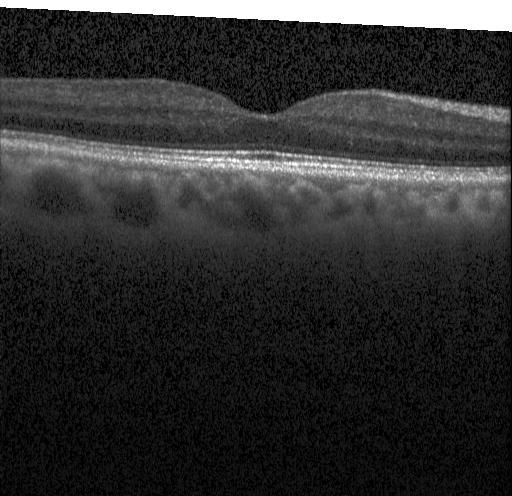

OCT B-scan showing neither CNV, DME, nor drusen.